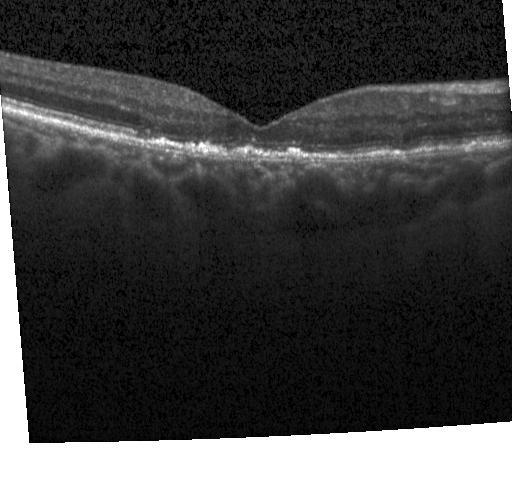
Finding: a choroidal neovascular membrane.